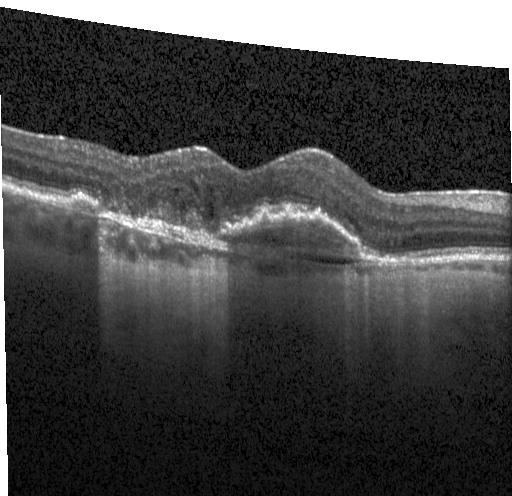 Retinal OCT cross-section showing a choroidal neovascular membrane.